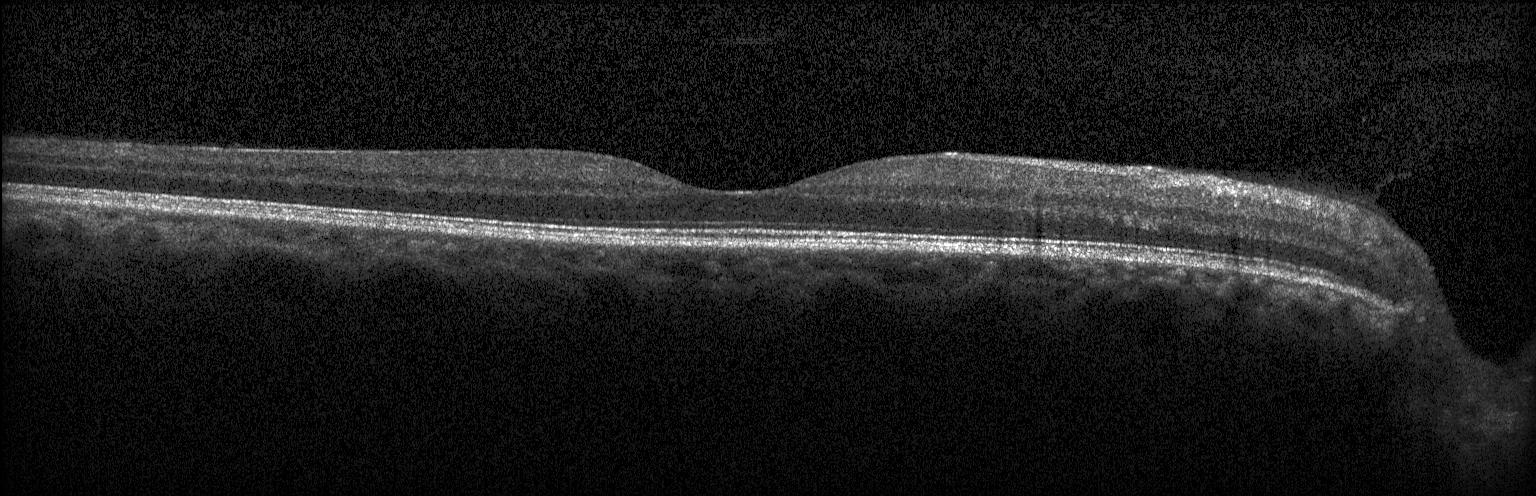

Horizontal scan through the fovea, acquired on a Heidelberg Spectralis, retinal OCT B-scan, spectral-domain OCT. No choroidal neovascularization, diabetic macular edema, or drusen.